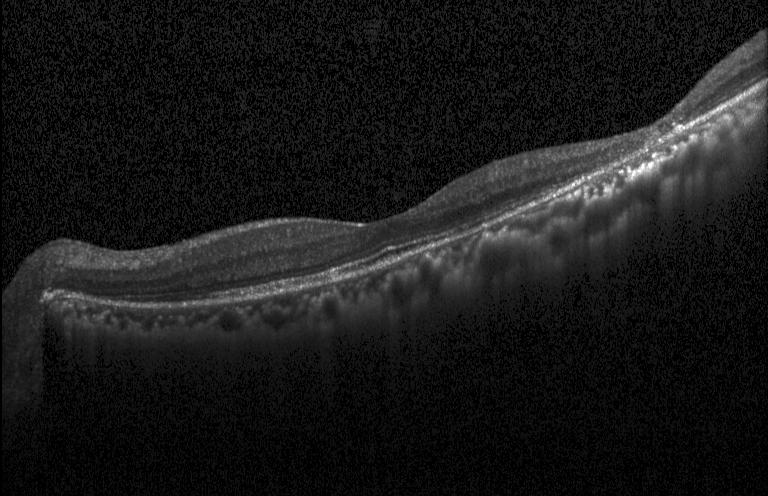 Finding: neither CNV, DME, nor drusen.